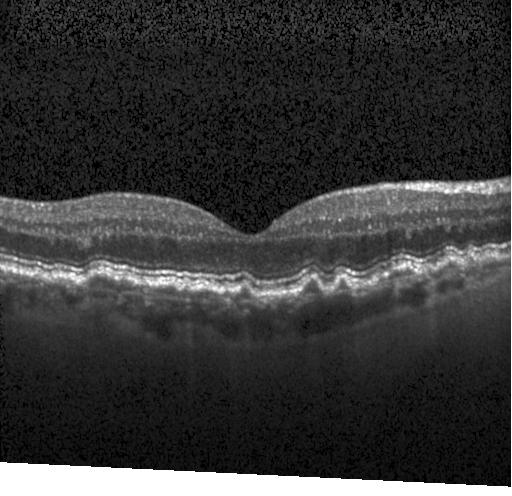

Finding: multiple drusen.